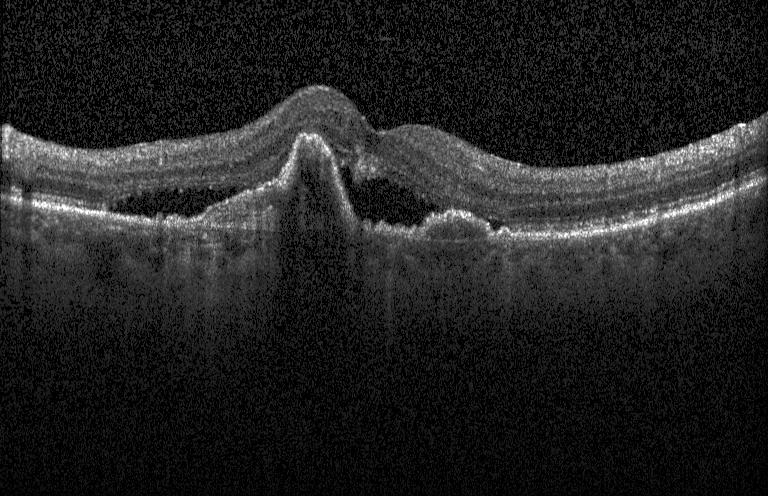
Diagnosis: CNV.